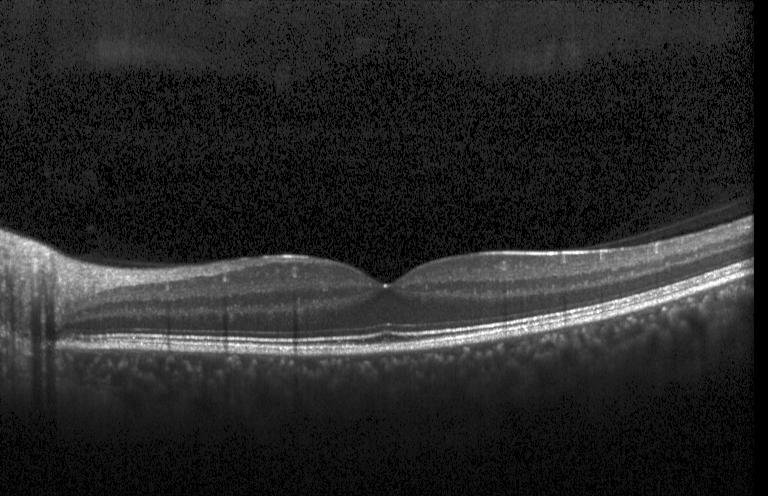

Optical coherence tomography scan. Acquired on a Heidelberg Spectralis. Spectral-domain OCT — The scan shows no choroidal neovascularization, diabetic macular edema, or drusen.